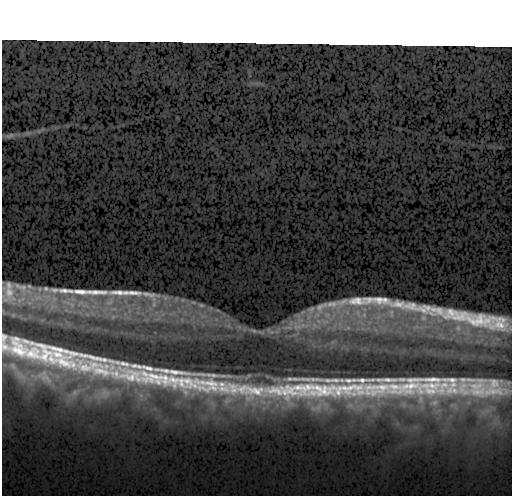
Retinal OCT cross-section showing no choroidal neovascularization, no diabetic macular edema, and no drusen.